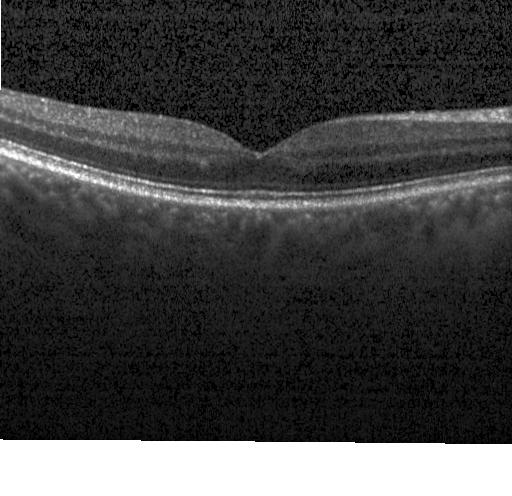
Through the macula; OCT B-scan.
The scan shows no choroidal neovascularization, no diabetic macular edema, and no drusen.